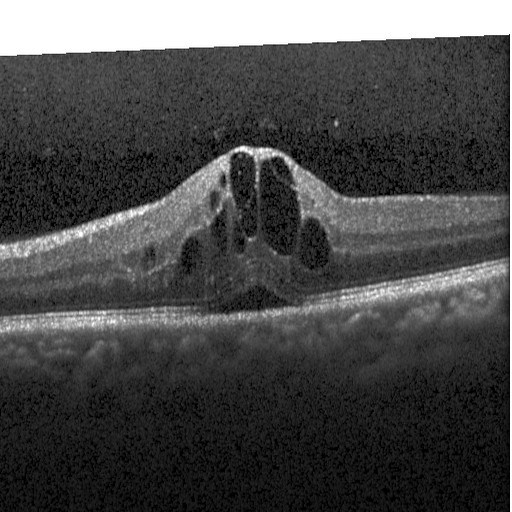

Dx: diabetic macular edema.